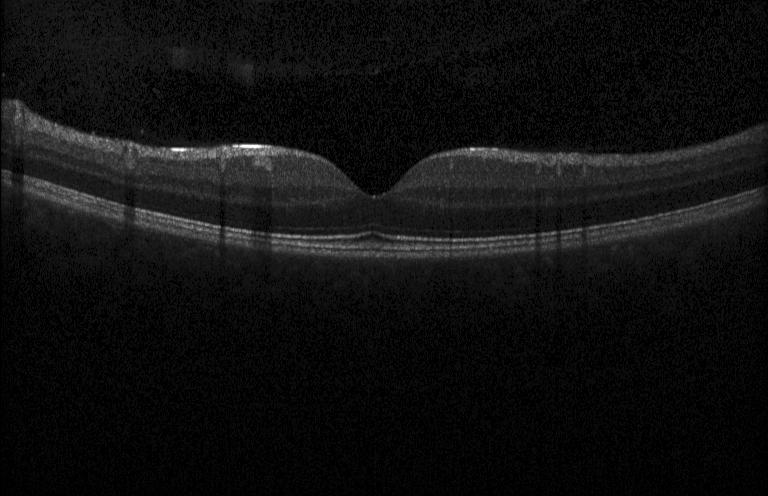

OCT B-scan — Finding: no CNV, no DME, and no drusen.